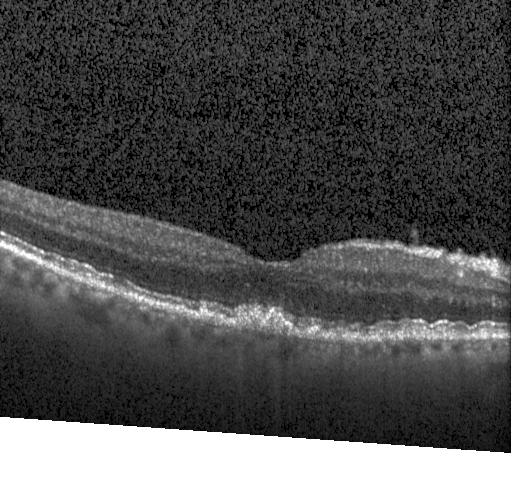

OCT line scan — The scan shows sub-RPE drusenoid deposits.